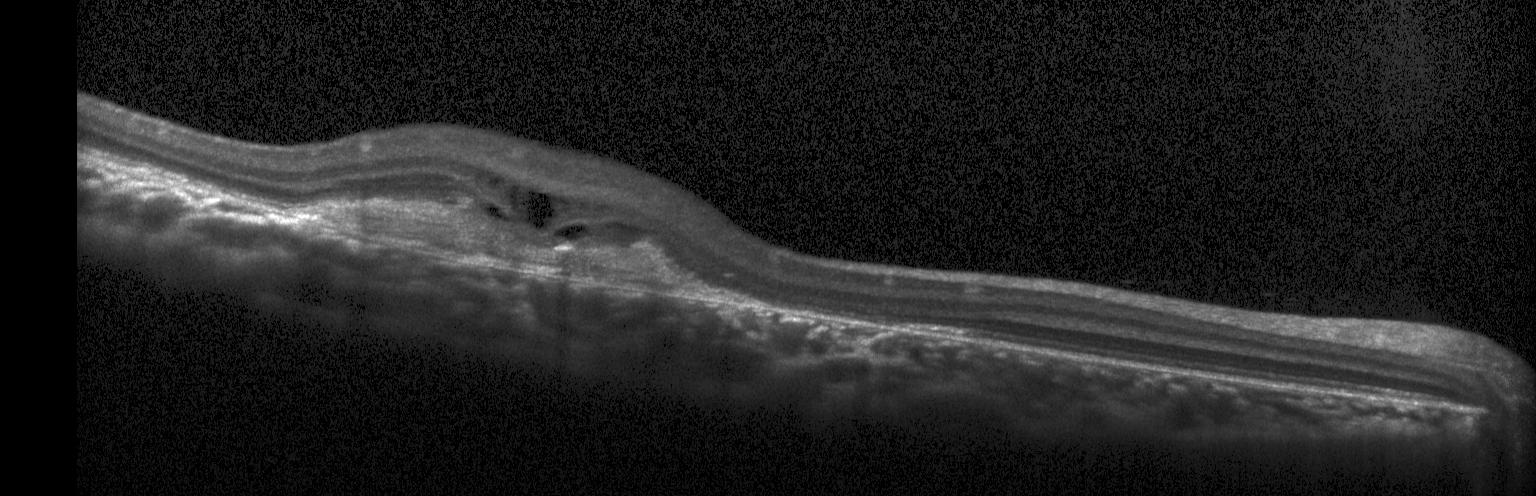 Spectral-domain OCT B-scan: a choroidal neovascular membrane.